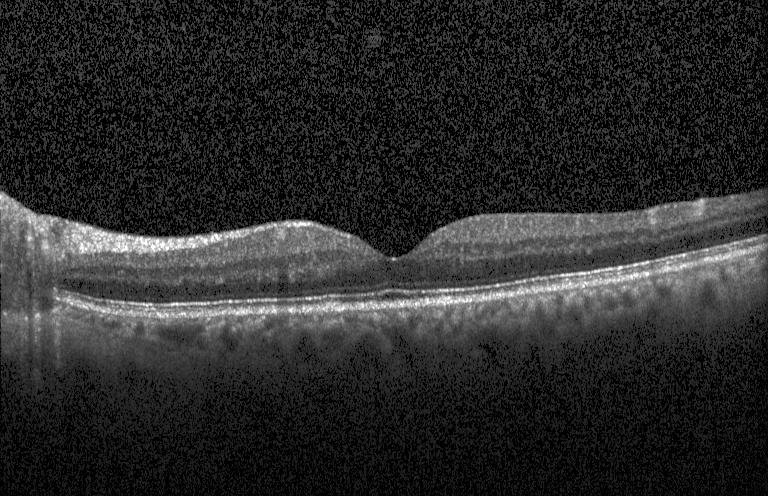
OCT scan showing no choroidal neovascularization, diabetic macular edema, or drusen.